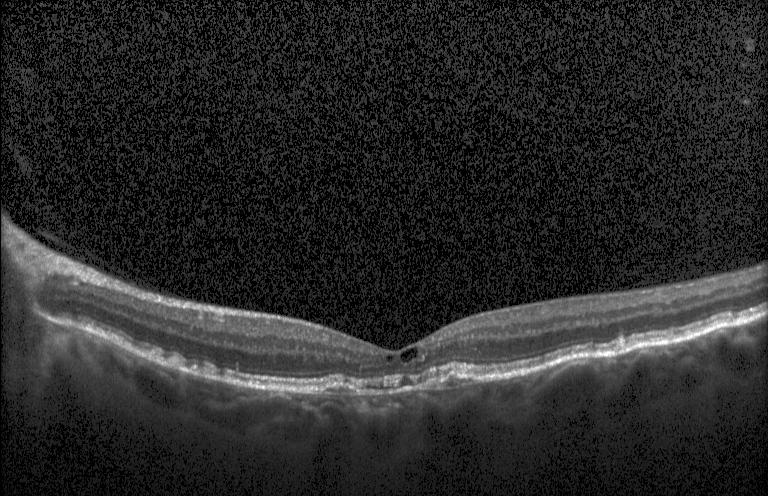

Diagnosis: choroidal neovascularization.